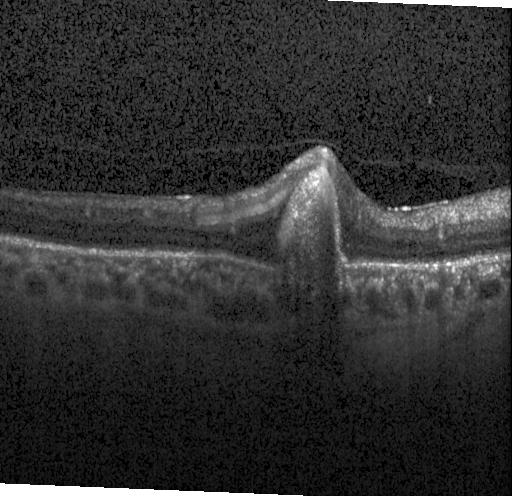
OCT B-scan showing CNV.